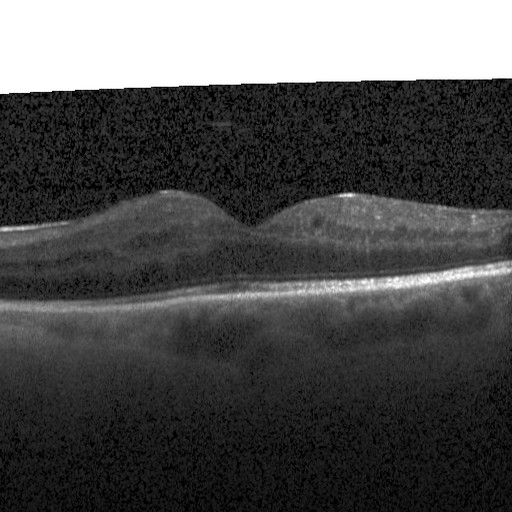

Dx: DME.